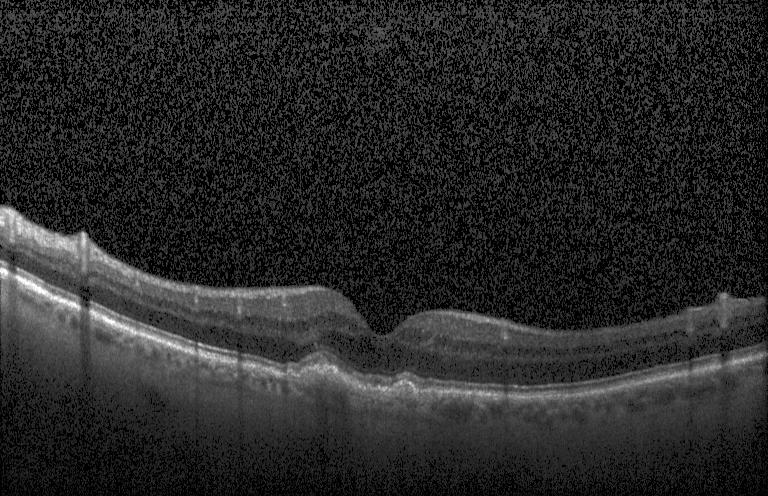
Impression: a choroidal neovascular membrane.